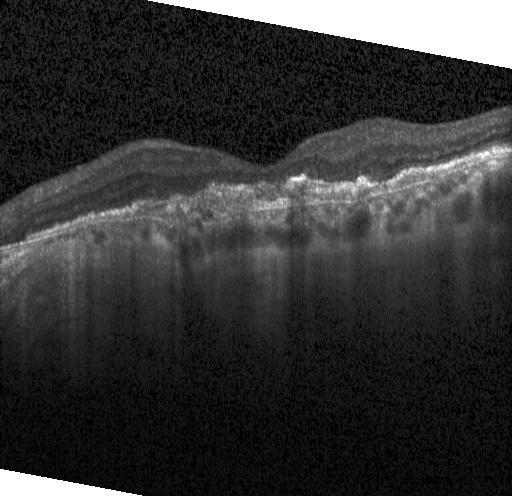 Optical coherence tomography scan — Macular OCT: CNV.